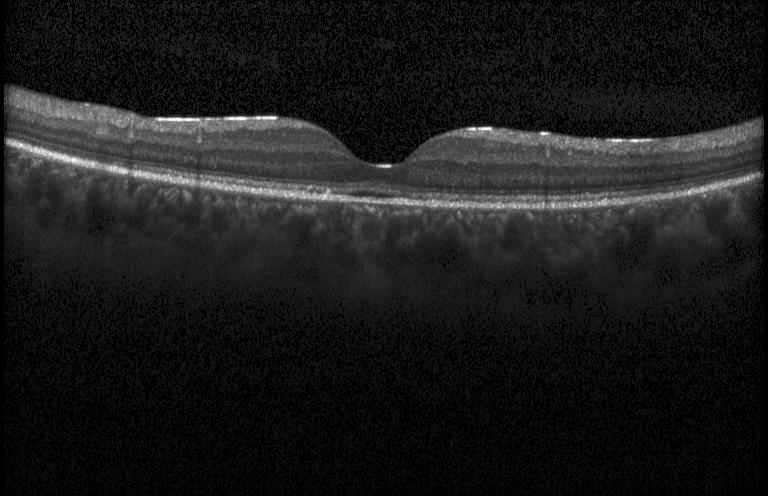
Macular OCT: no choroidal neovascularization, diabetic macular edema, or drusen.